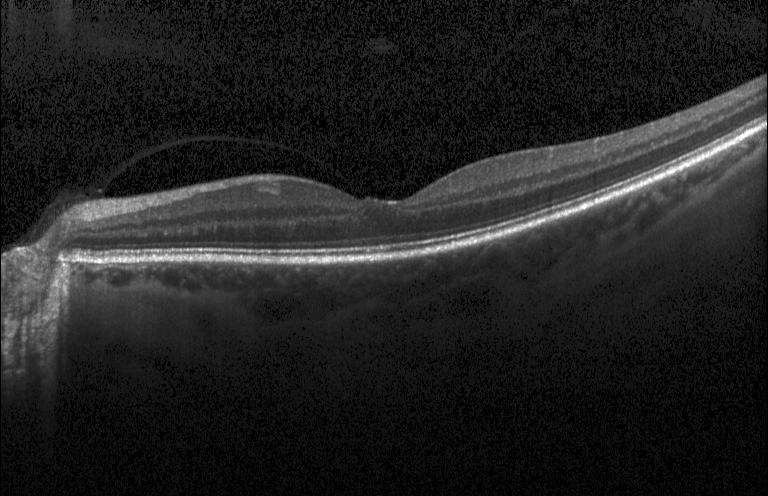
Retinal OCT B-scan, Heidelberg Spectralis, fovea-centered, spectral-domain OCT.
OCT finding: no choroidal neovascularization, diabetic macular edema, or drusen.